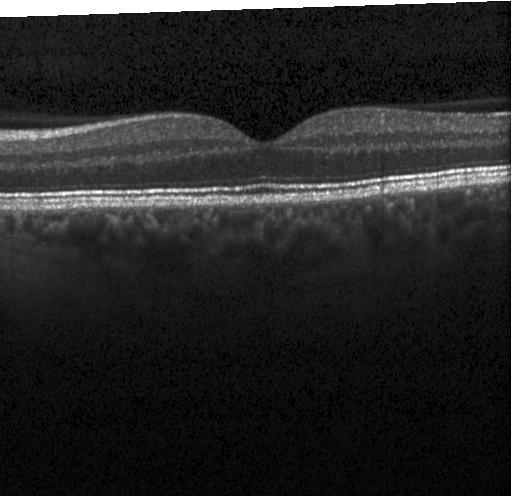

Finding: neither choroidal neovascularization, diabetic macular edema, nor drusen.